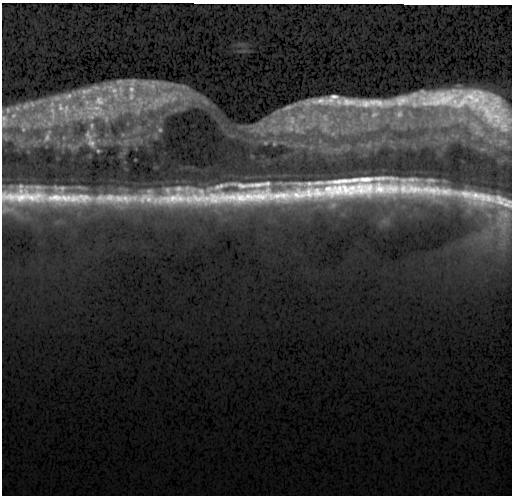 Optical coherence tomography scan; instrument: Heidelberg Spectralis; spectral-domain OCT.
Finding: DME.